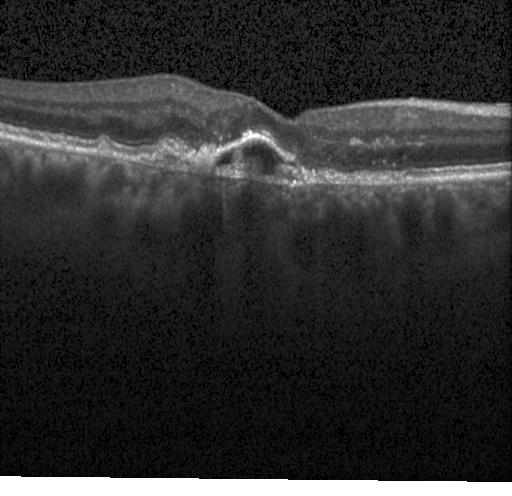

Spectral-domain optical coherence tomography. OCT B-scan. Acquired on a Heidelberg Spectralis
OCT finding: choroidal neovascularization.